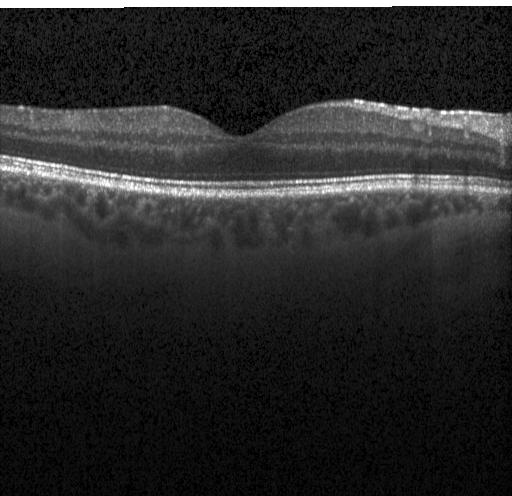 Retinal OCT cross-section; instrument: Heidelberg Spectralis; through the macula; spectral-domain OCT — Assessment: no CNV, no DME, and no drusen.